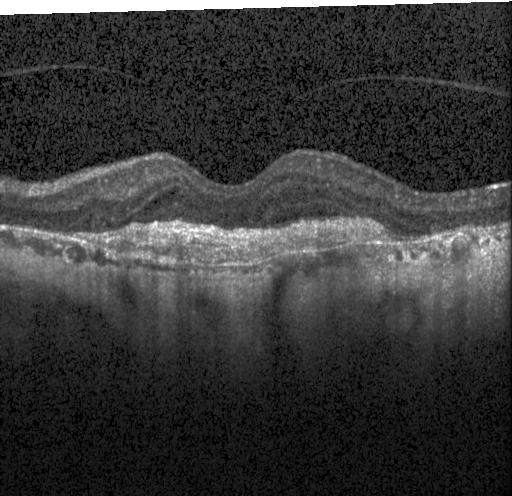

Macular OCT: a choroidal neovascular membrane.